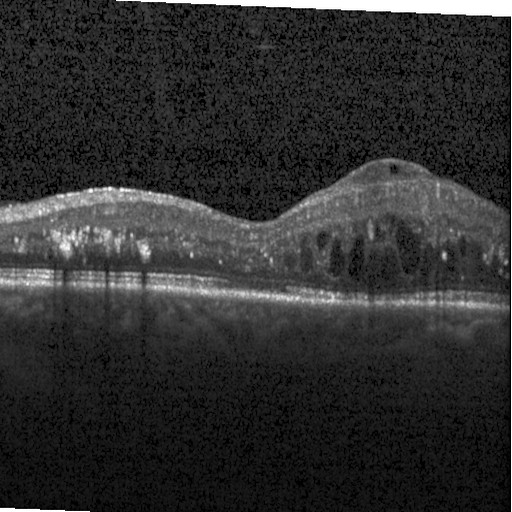
Optical coherence tomography scan, spectral-domain OCT, fovea-centered — Diagnosis: diabetic macular edema.